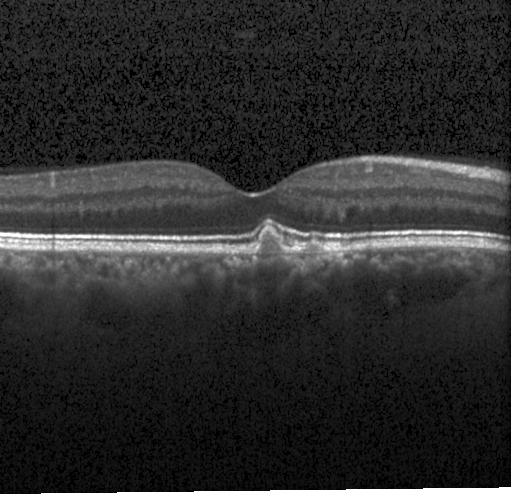
Macular OCT demonstrating drusen.